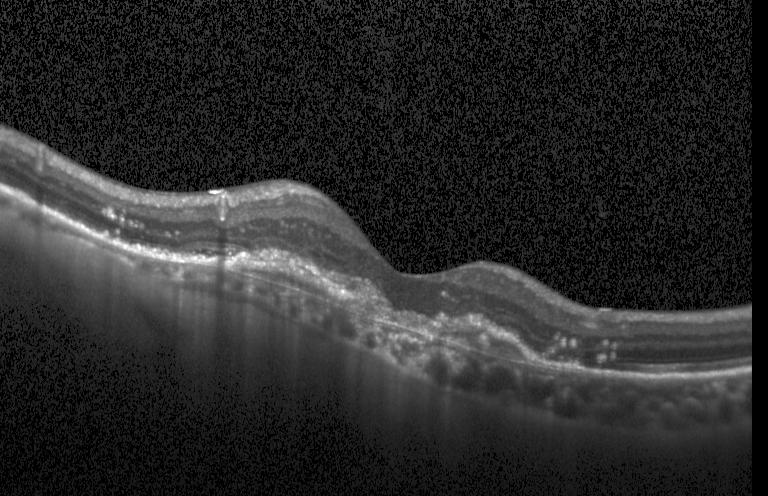
OCT line scan. Assessment: a choroidal neovascular membrane.